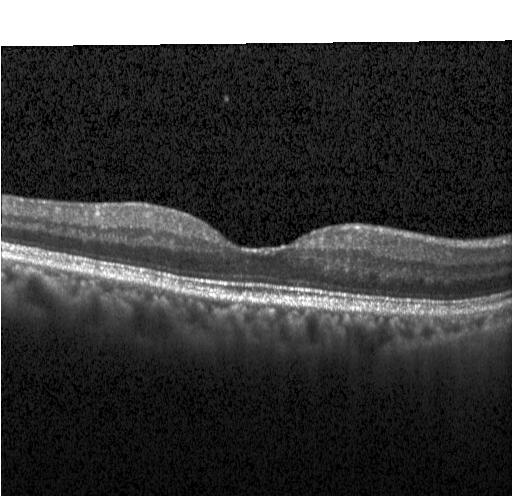

Assessment: neither choroidal neovascularization, diabetic macular edema, nor drusen.